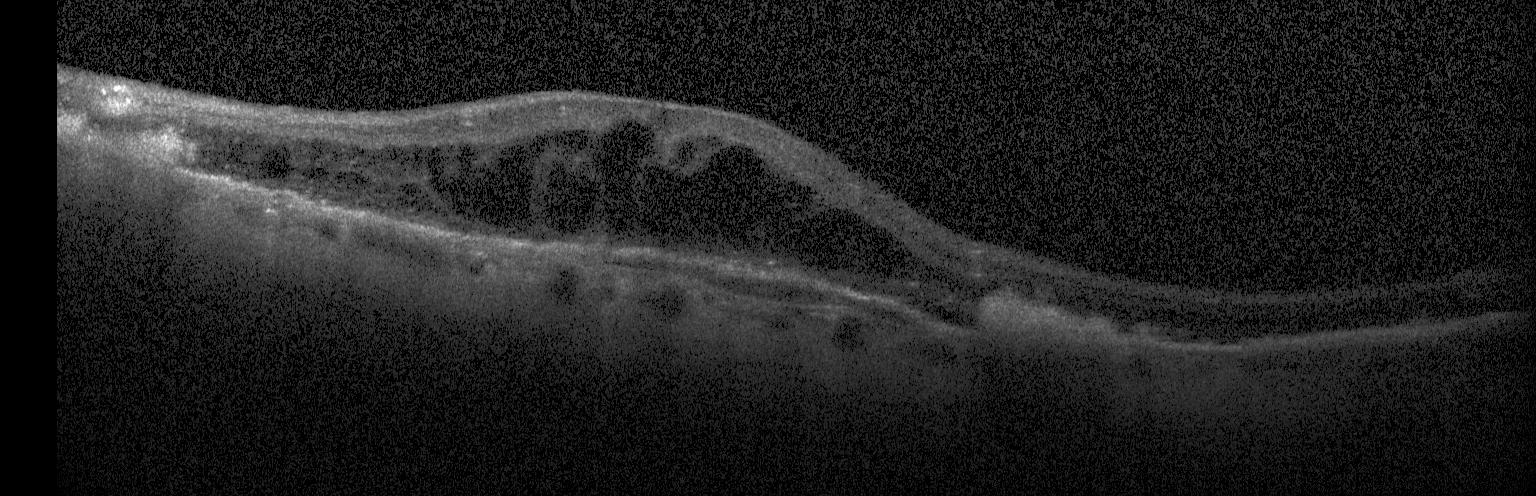

OCT scan showing CNV.